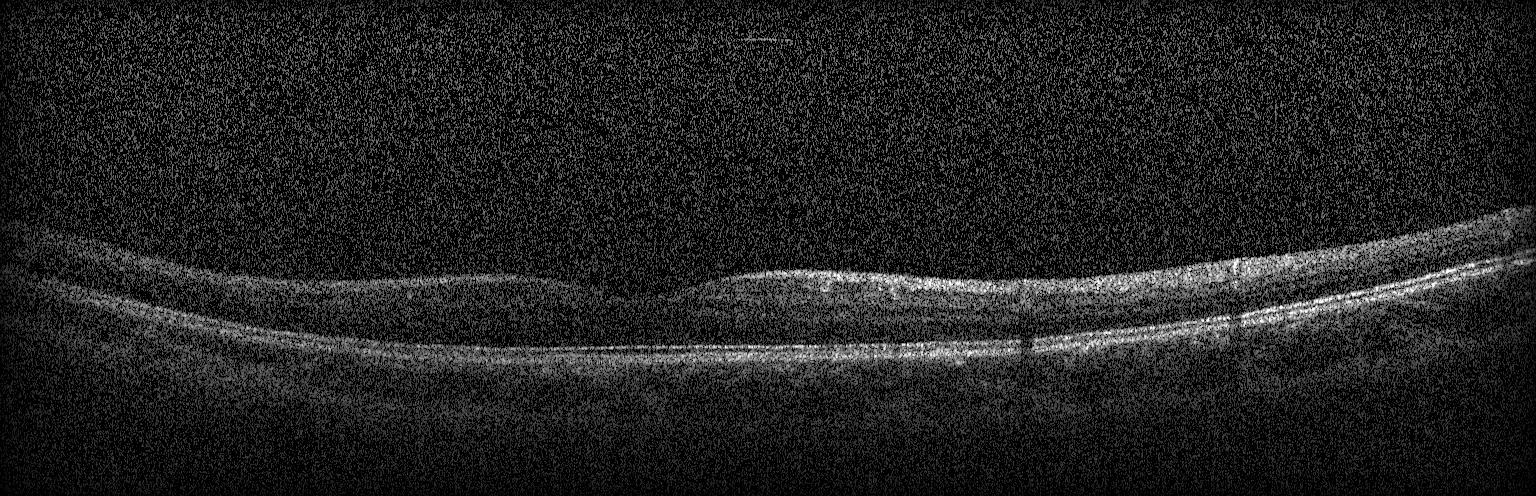
OCT line scan; through the macula; Heidelberg Spectralis OCT system; spectral-domain OCT — Assessment: neither CNV, DME, nor drusen.